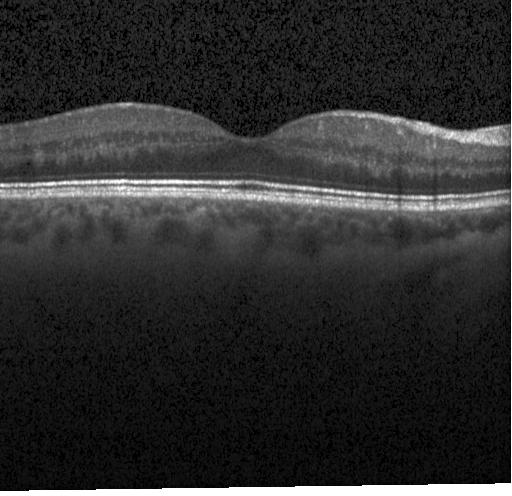

Spectral-domain optical coherence tomography, OCT line scan, instrument: Heidelberg Spectralis — Dx: no CNV, no DME, and no drusen.